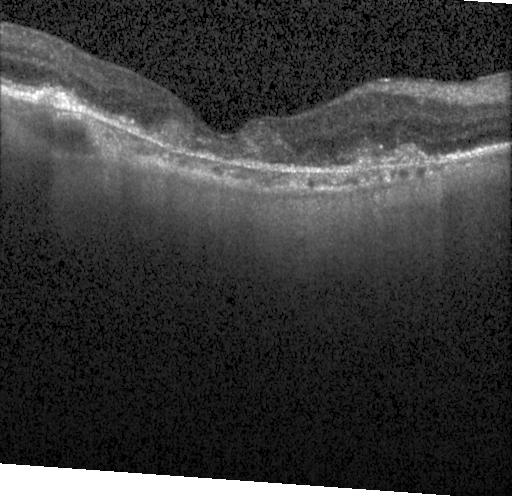

Finding: a choroidal neovascular membrane.